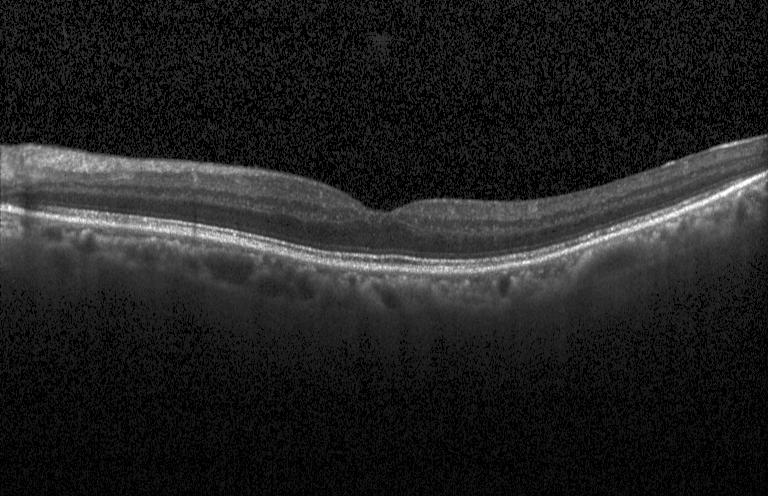
Centered on the fovea. Optical coherence tomography B-scan. Heidelberg Spectralis OCT system. Spectral-domain optical coherence tomography — Impression: no choroidal neovascularization, diabetic macular edema, or drusen.